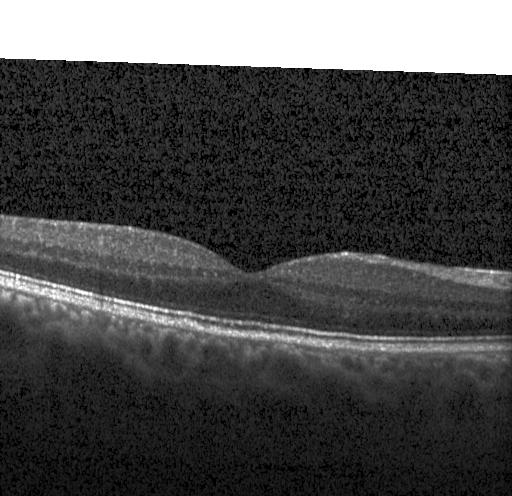
Finding: no choroidal neovascularization, diabetic macular edema, or drusen.